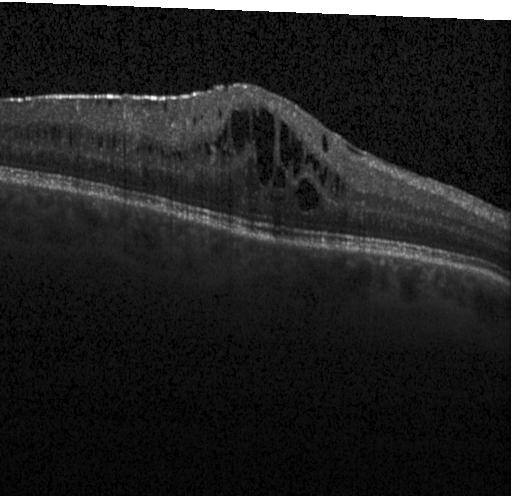

Diagnosis: diabetic macular edema (DME).